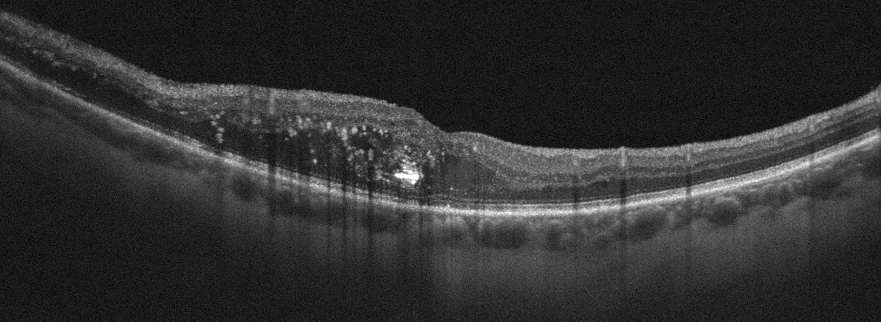 OCT line scan · fovea-centered · Optovue Avanti RTVue XR — Impression: DME.